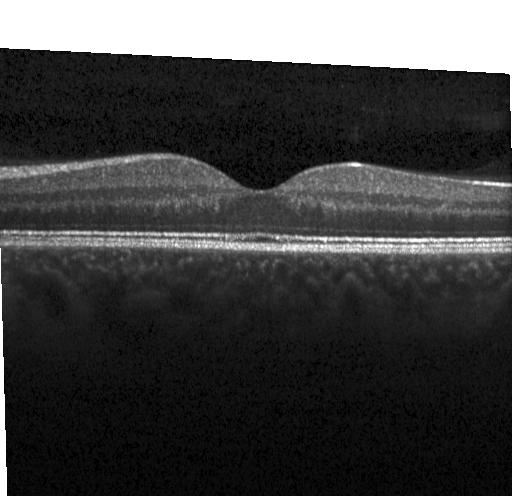

Retinal OCT cross-section showing no CNV, DME, or drusen.